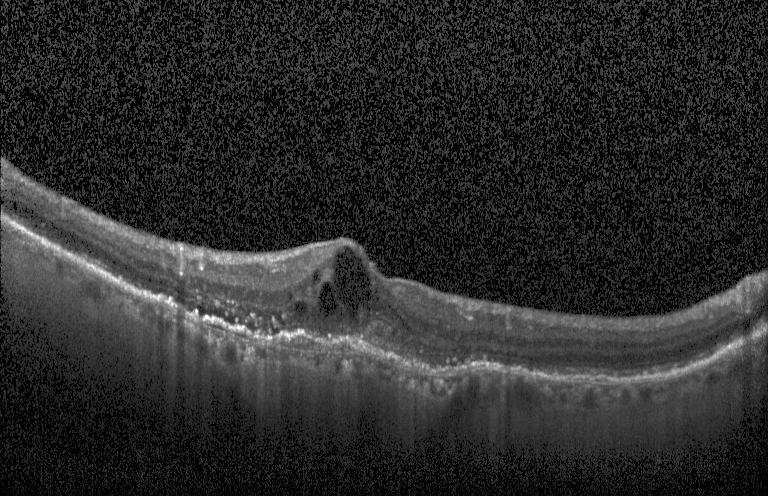
Retinal OCT cross-section. OCT finding: choroidal neovascularization.